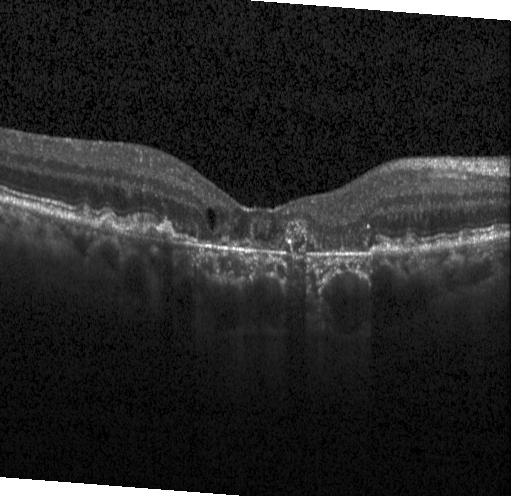 Optical coherence tomography B-scan · acquired on a Heidelberg Spectralis · centered on the fovea · SD-OCT.
Impression: choroidal neovascularization (CNV).